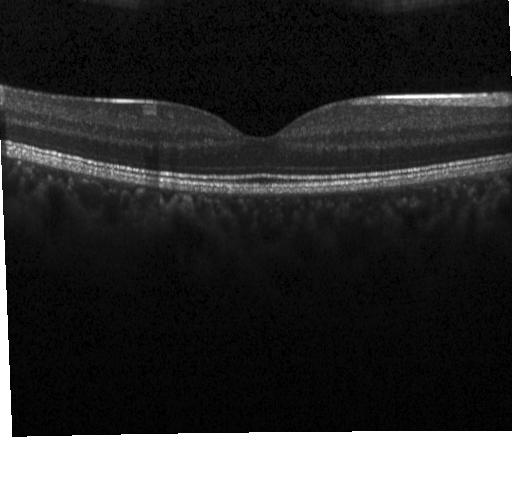 Spectral-domain optical coherence tomography · retinal OCT cross-section · horizontal scan through the fovea.
Diagnosis: no choroidal neovascularization, no diabetic macular edema, and no drusen.